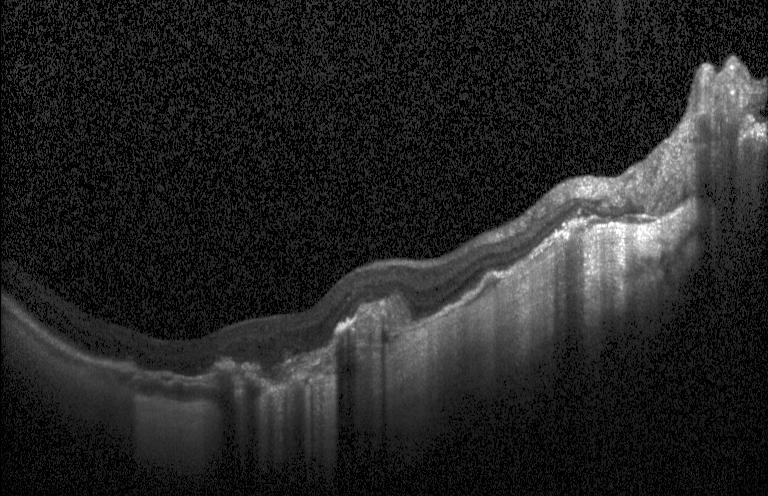 Optical coherence tomography B-scan — Finding: a choroidal neovascular membrane.